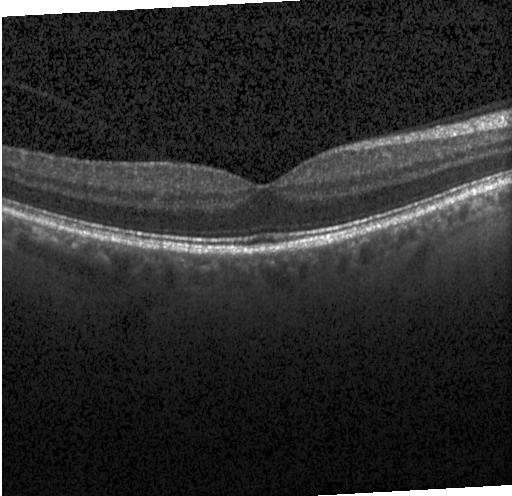 Optical coherence tomography B-scan, SD-OCT, horizontal scan through the fovea.
Macular OCT: no CNV, DME, or drusen.